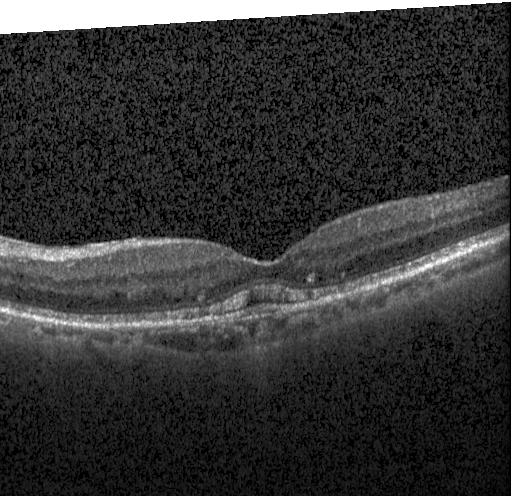

Optical coherence tomography scan. Fovea-centered. SD-OCT. Acquired on a Heidelberg Spectralis — Finding: choroidal neovascularization (CNV).